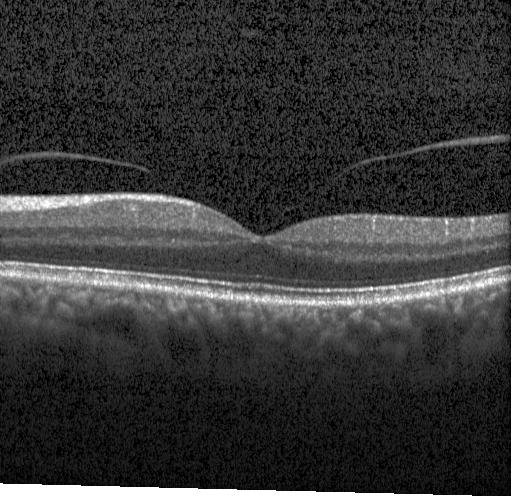 Optical coherence tomography B-scan · SD-OCT · centered on the fovea · acquired on a Heidelberg Spectralis — Finding: neither choroidal neovascularization, diabetic macular edema, nor drusen.